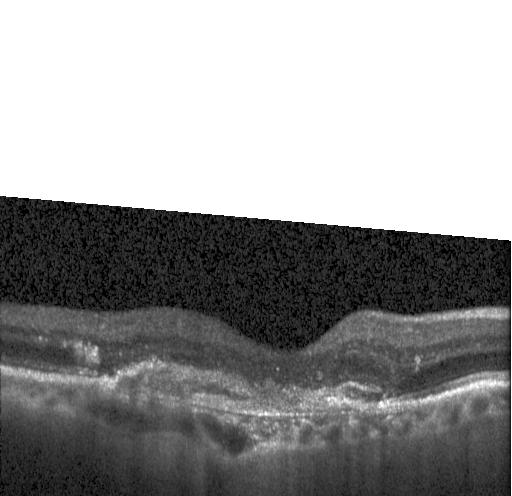 OCT finding: choroidal neovascularization (CNV).